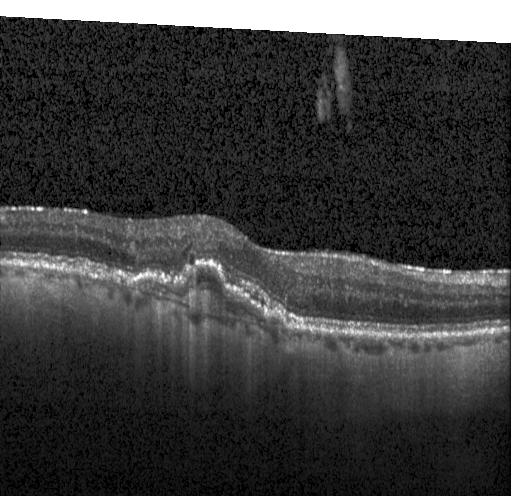 Retinal OCT B-scan. Heidelberg Spectralis. Centered on the fovea.
Diagnosis: choroidal neovascularization (CNV).